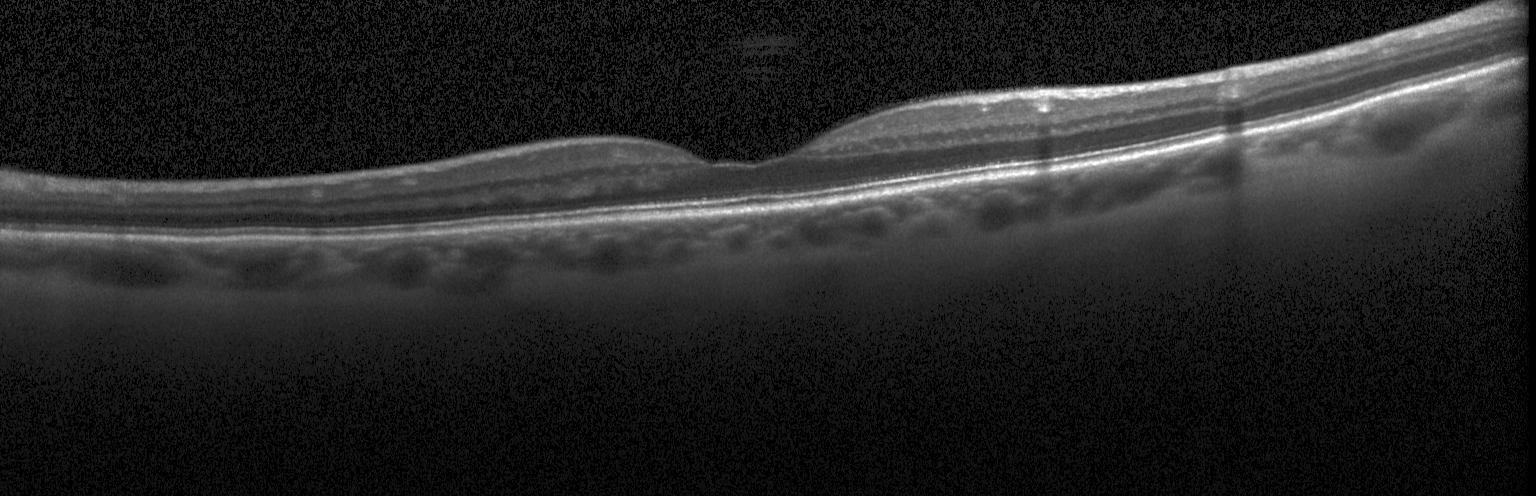 Spectral-domain OCT. Retinal OCT cross-section. Instrument: Heidelberg Spectralis — Dx: neither CNV, DME, nor drusen.